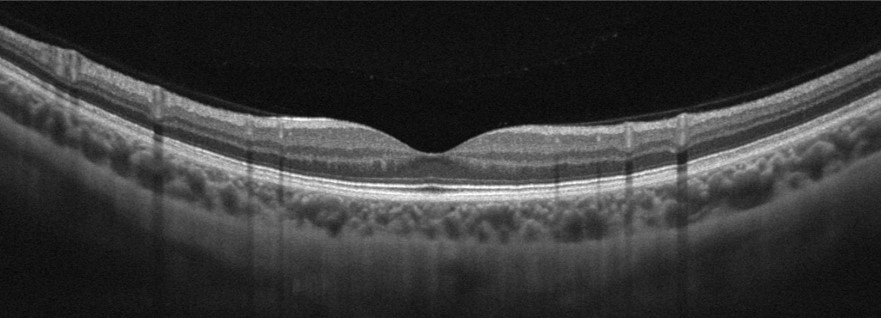 Assessment: no AMD, DME, ERM, RAO, RVO, or VID.